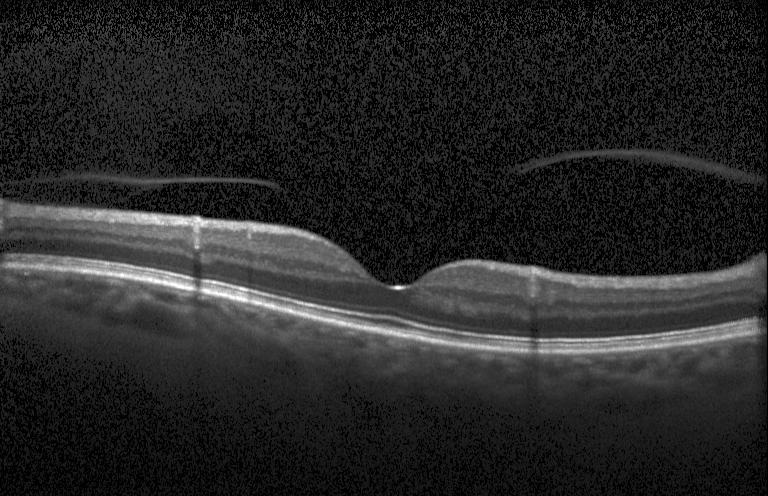 SD-OCT; fovea-centered; optical coherence tomography B-scan; instrument: Heidelberg Spectralis. Impression: no evidence of choroidal neovascularization, diabetic macular edema, or drusen.